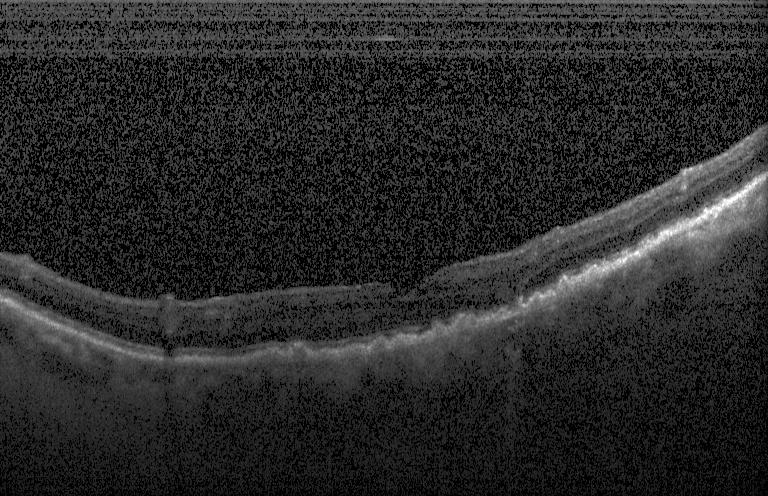
Optical coherence tomography B-scan · spectral-domain optical coherence tomography.
OCT finding: multiple drusen.